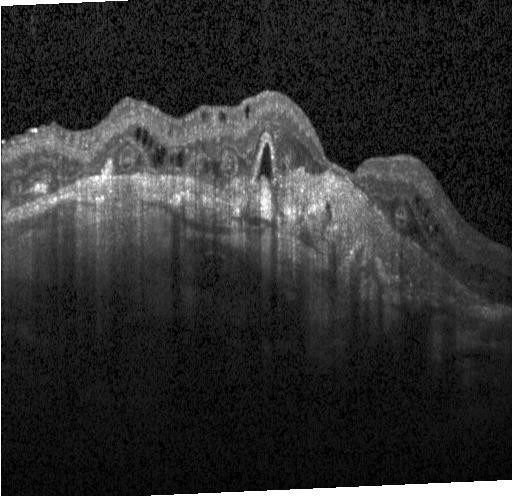
Spectral-domain OCT, optical coherence tomography B-scan.
Diagnosis: a choroidal neovascular membrane.